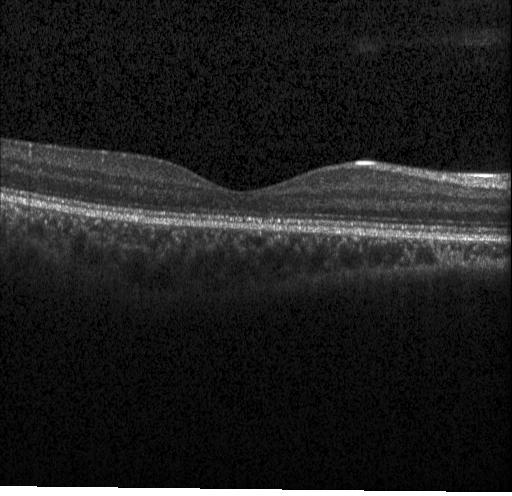

Acquired on a Heidelberg Spectralis · fovea-centered · OCT B-scan · SD-OCT
Impression: neither choroidal neovascularization, diabetic macular edema, nor drusen.